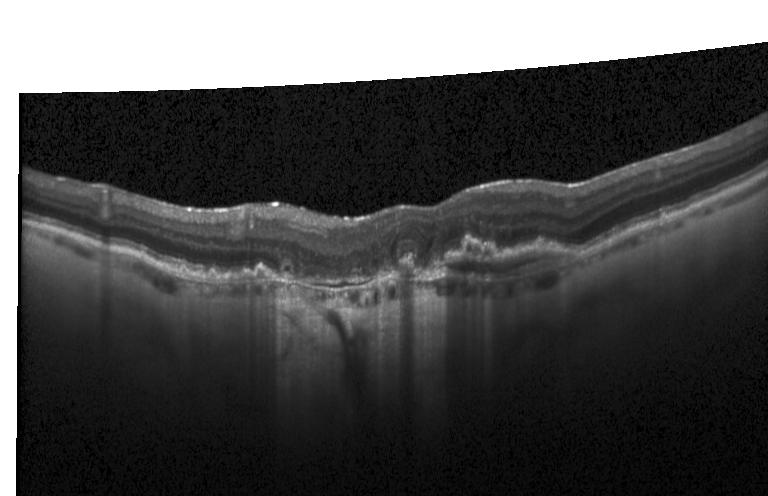

Impression: choroidal neovascularization.